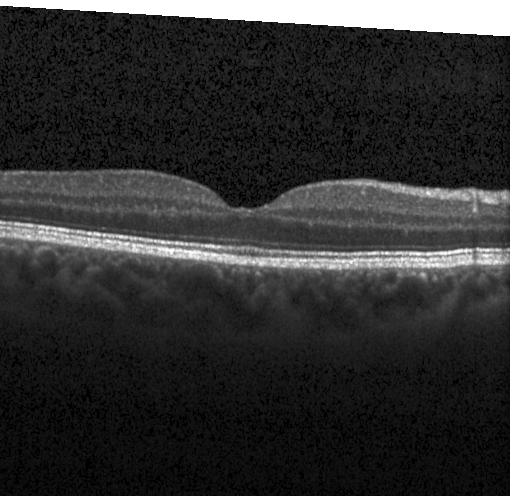

OCT line scan, macular scan
Impression: neither CNV, DME, nor drusen.